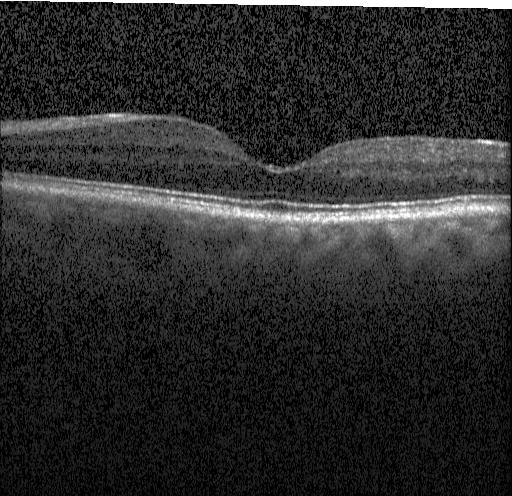
Heidelberg Spectralis OCT system, centered on the fovea, SD-OCT, retinal OCT B-scan
Diagnosis: neither CNV, DME, nor drusen.